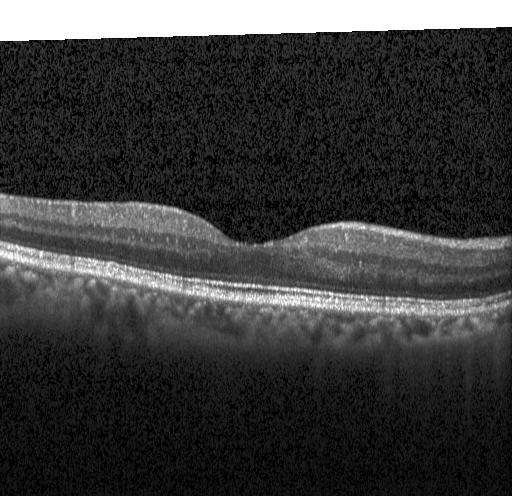

OCT line scan · SD-OCT · centered on the fovea. Diagnosis: no evidence of choroidal neovascularization, diabetic macular edema, or drusen.